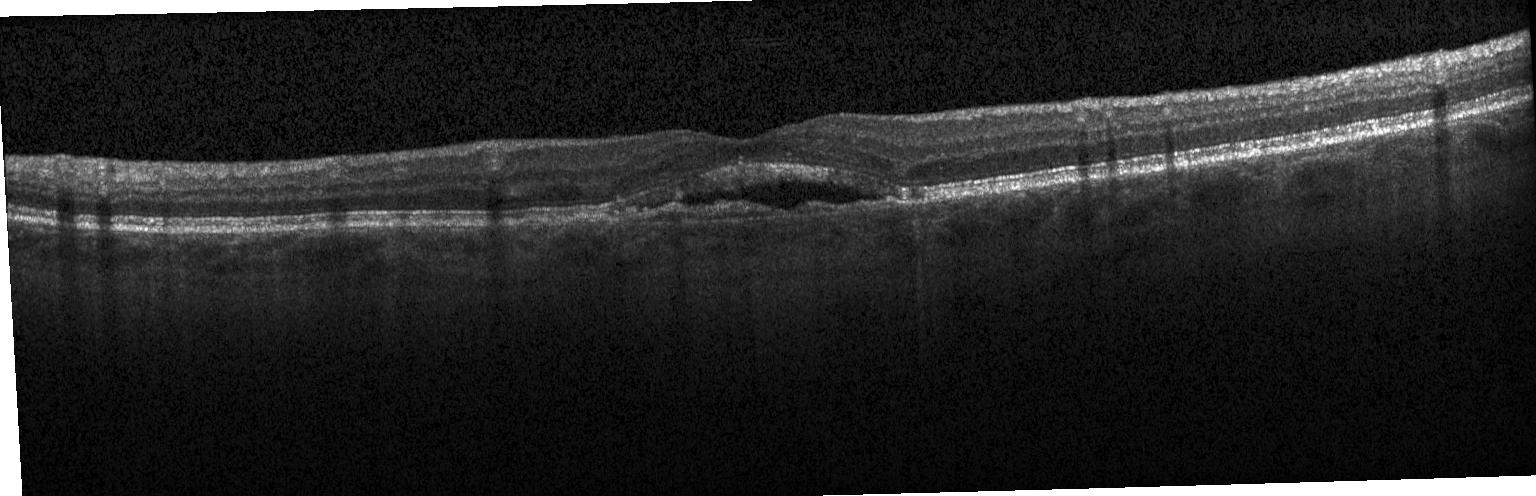 This B-scan demonstrates a choroidal neovascular membrane.